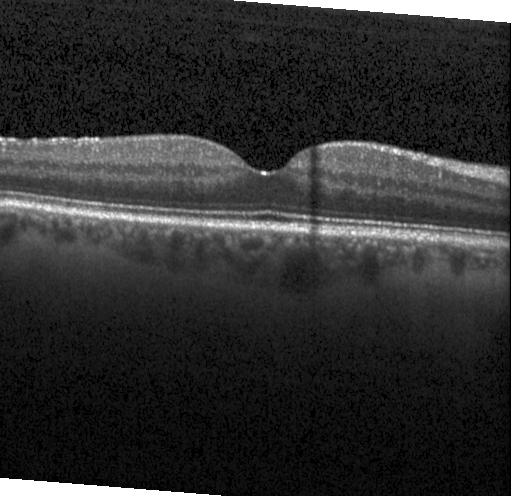 Dx: no choroidal neovascularization, diabetic macular edema, or drusen.